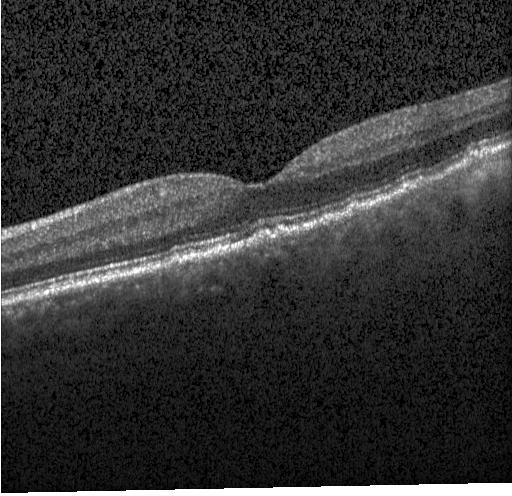 Impression: drusen.